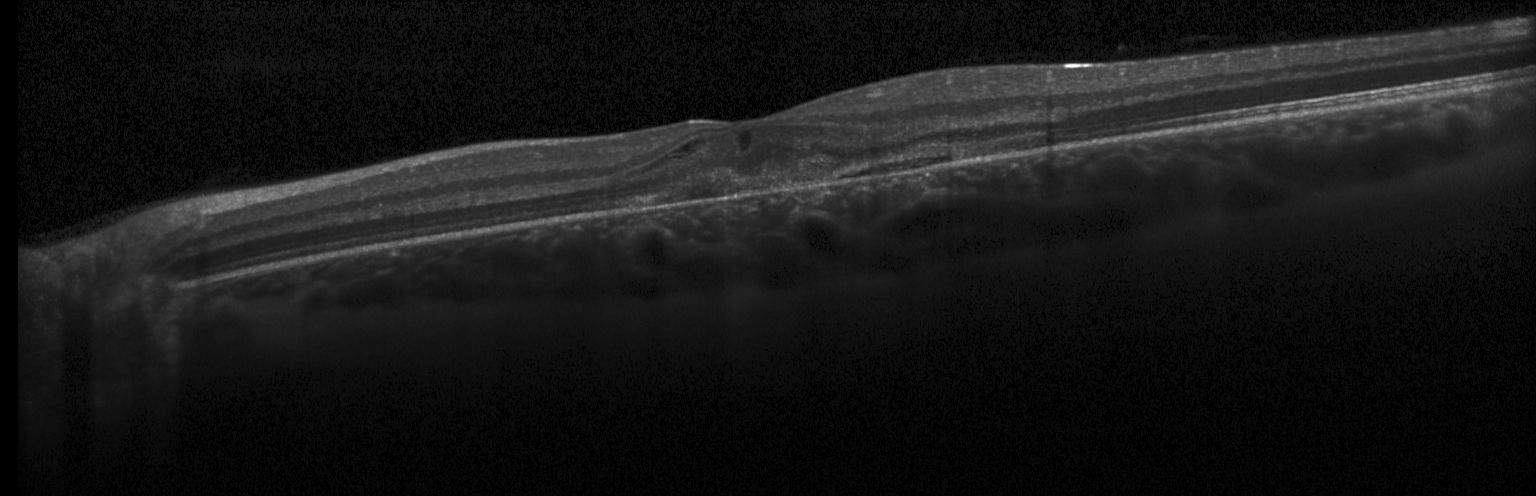
Dx: a choroidal neovascular membrane.